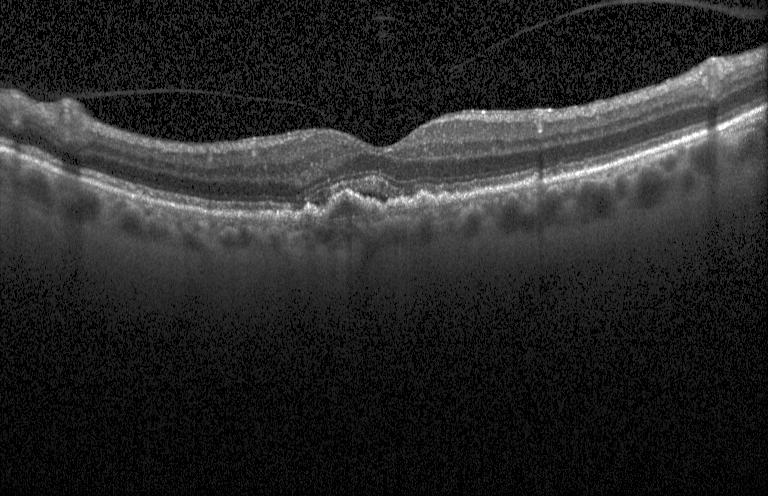

Horizontal scan through the fovea · spectral-domain OCT · instrument: Heidelberg Spectralis · optical coherence tomography B-scan
Assessment: choroidal neovascularization.